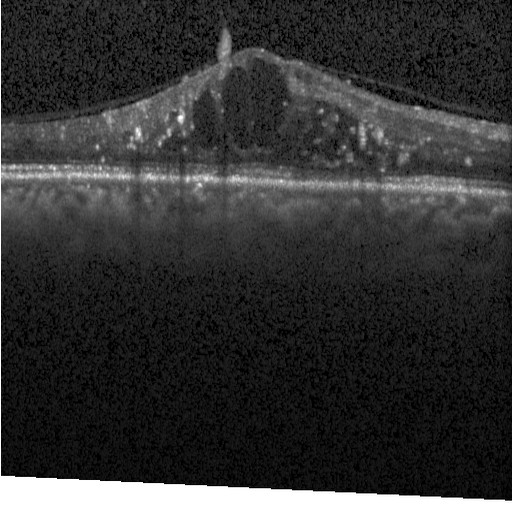

Horizontal scan through the fovea, Heidelberg Spectralis, SD-OCT, optical coherence tomography scan.
Impression: diabetic macular edema.